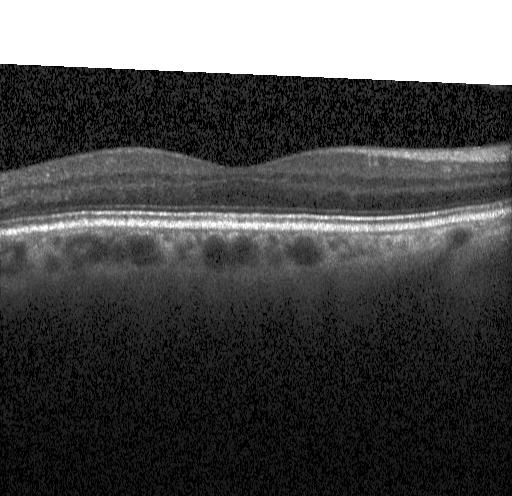
OCT line scan. Horizontal scan through the fovea
Impression: neither CNV, DME, nor drusen.